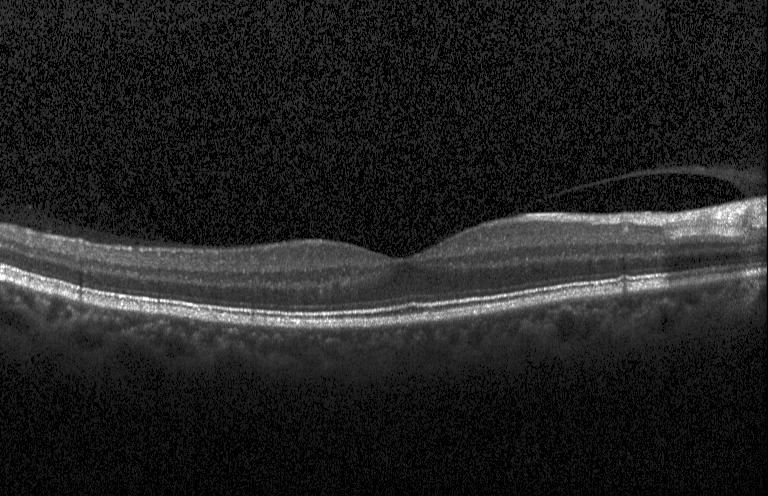 Acquired on a Heidelberg Spectralis; retinal OCT cross-section; centered on the fovea — Impression: no CNV, DME, or drusen.